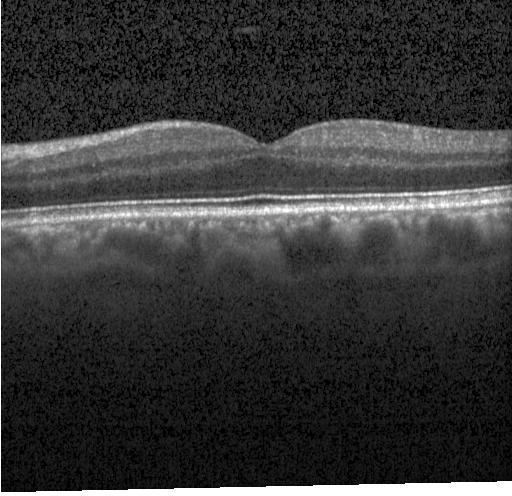

Assessment: neither choroidal neovascularization, diabetic macular edema, nor drusen.